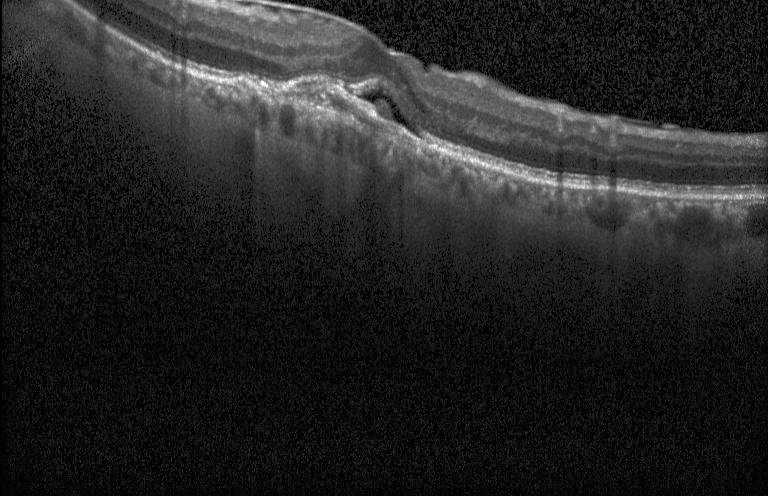

Horizontal scan through the fovea; retinal OCT cross-section. Dx: CNV.